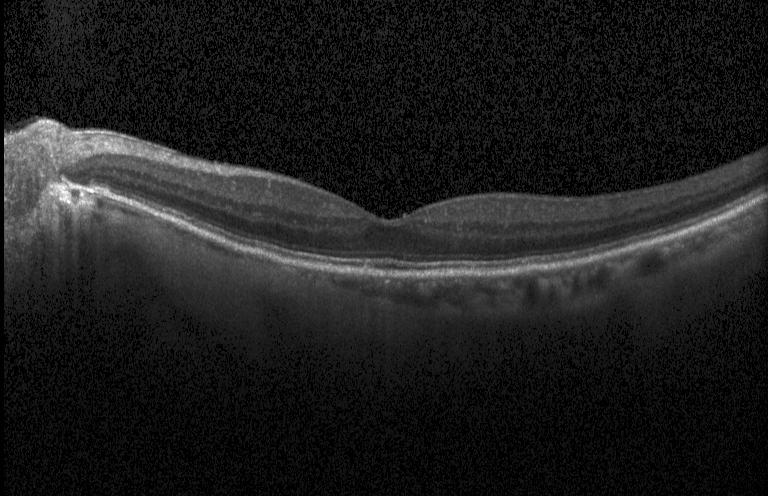
Optical coherence tomography scan · centered on the fovea. The scan shows no choroidal neovascularization, no diabetic macular edema, and no drusen.